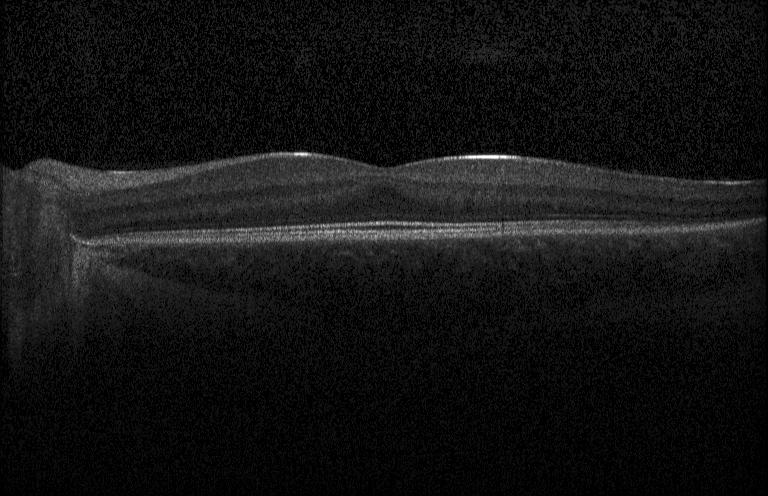 Heidelberg Spectralis · fovea-centered · spectral-domain optical coherence tomography · optical coherence tomography scan
Diagnosis: no evidence of choroidal neovascularization, diabetic macular edema, or drusen.